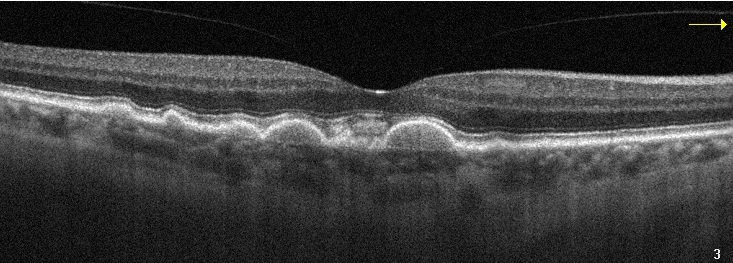 Macular OCT demonstrating age-related macular degeneration (AMD).